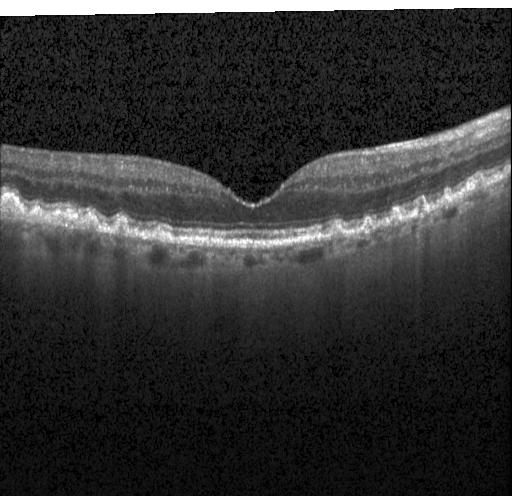 Horizontal scan through the fovea, OCT B-scan.
Finding: drusen.